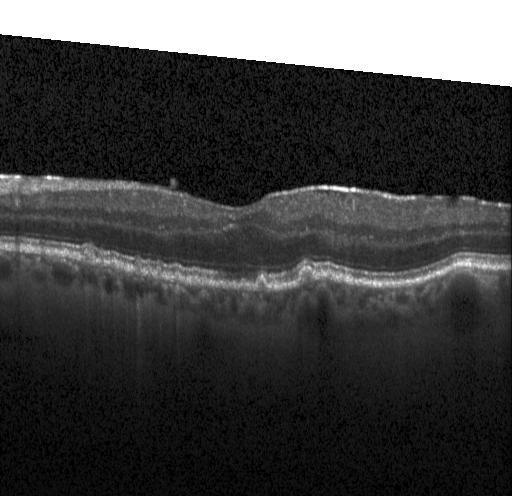
Spectral-domain OCT; retinal OCT cross-section
Finding: sub-RPE drusenoid deposits.